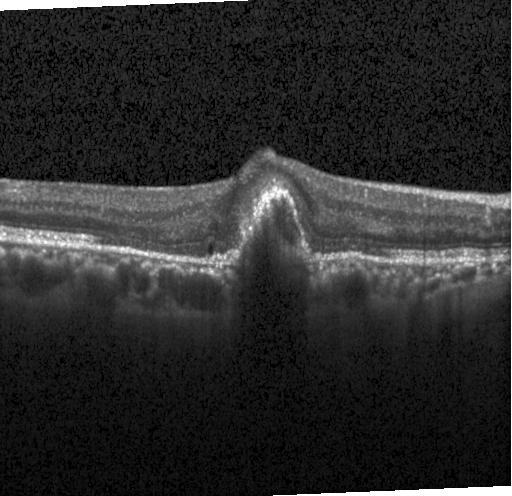
Finding: choroidal neovascularization (CNV).